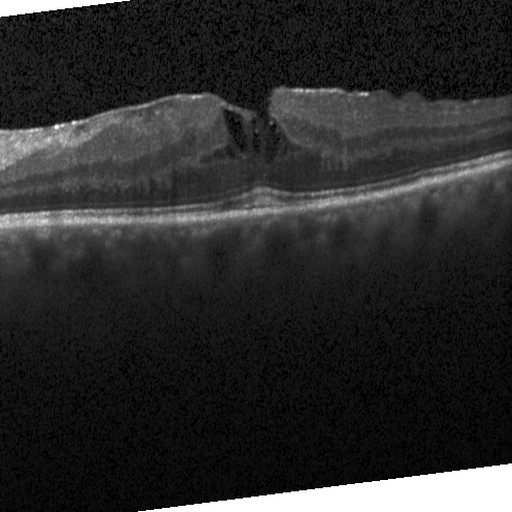

Centered on the fovea · spectral-domain optical coherence tomography · retinal OCT cross-section · acquired on a Heidelberg Spectralis.
Diagnosis: DME.